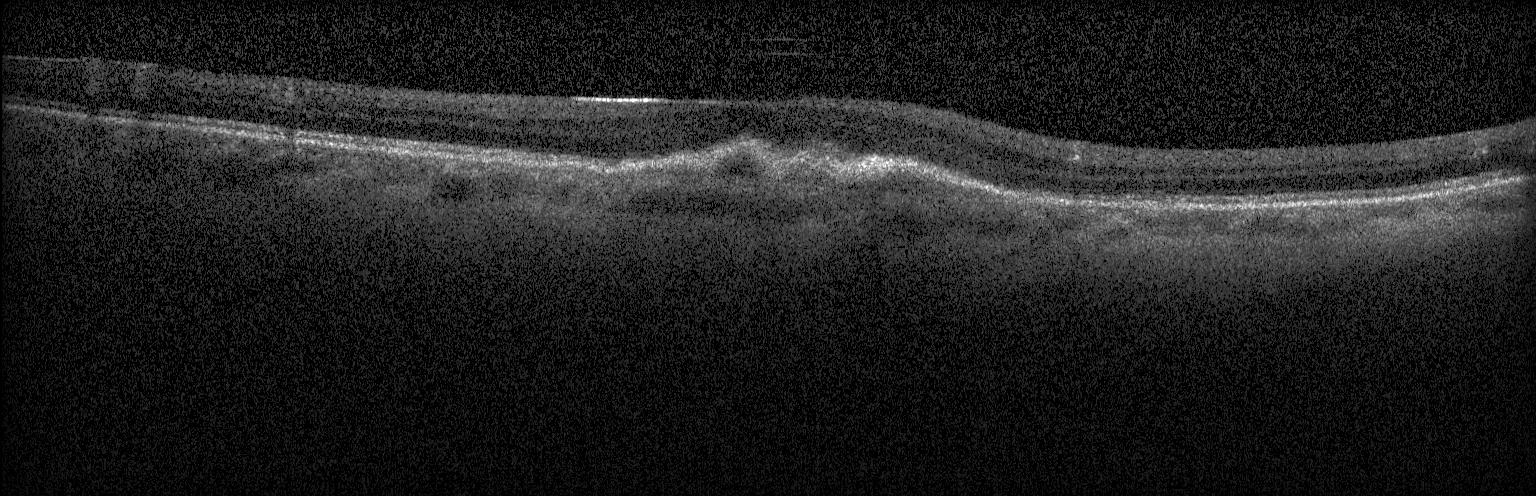

Spectral-domain optical coherence tomography. Optical coherence tomography B-scan. This B-scan demonstrates choroidal neovascularization (CNV).